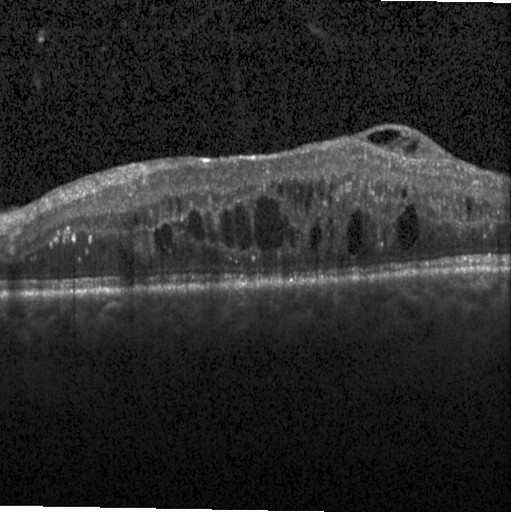 Assessment: diabetic macular edema (DME).